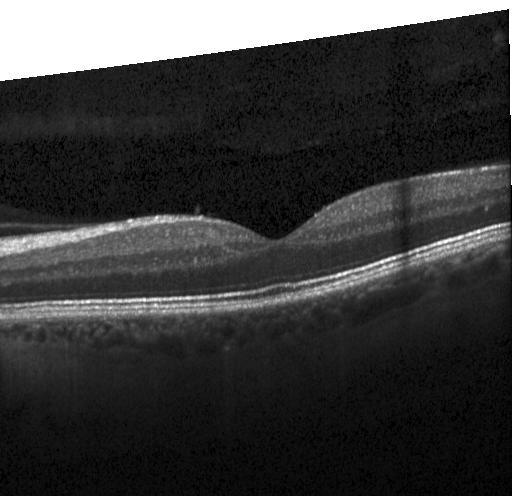

Heidelberg Spectralis, horizontal scan through the fovea, retinal OCT B-scan, spectral-domain OCT
Impression: no choroidal neovascularization, diabetic macular edema, or drusen.